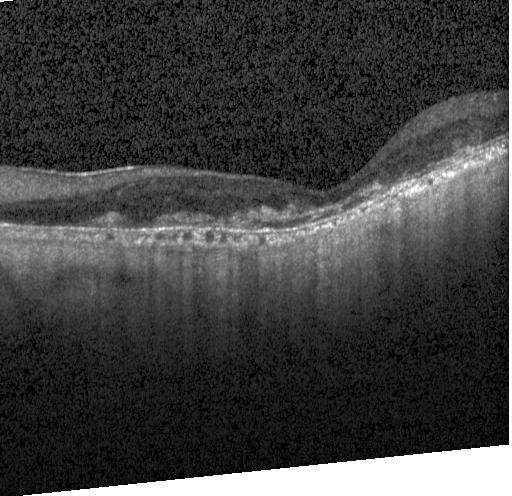 OCT finding: CNV.